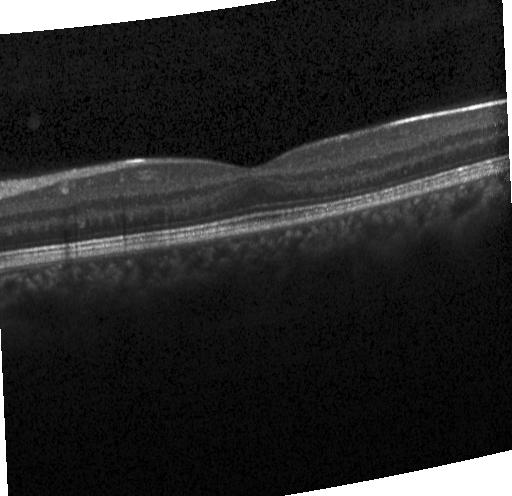 Optical coherence tomography scan. SD-OCT — This B-scan demonstrates neither CNV, DME, nor drusen.